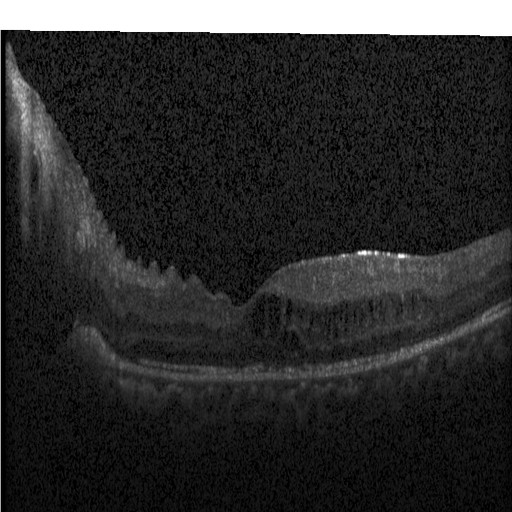 Finding: diabetic macular edema.